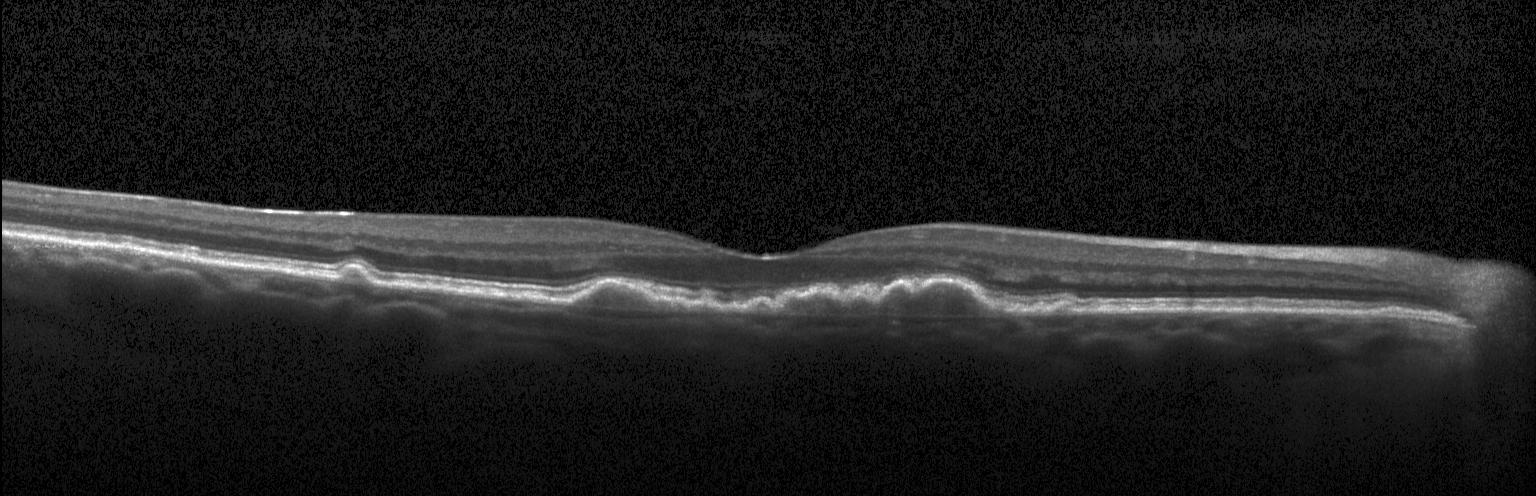 Macular OCT: multiple drusen.